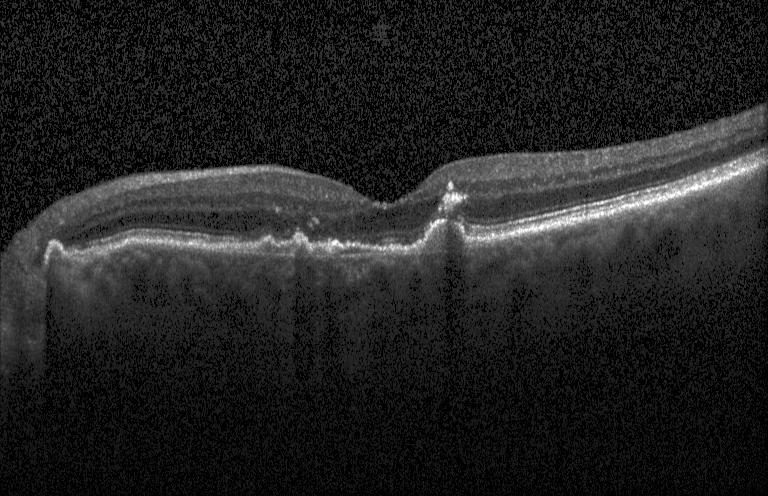

A choroidal neovascular membrane.